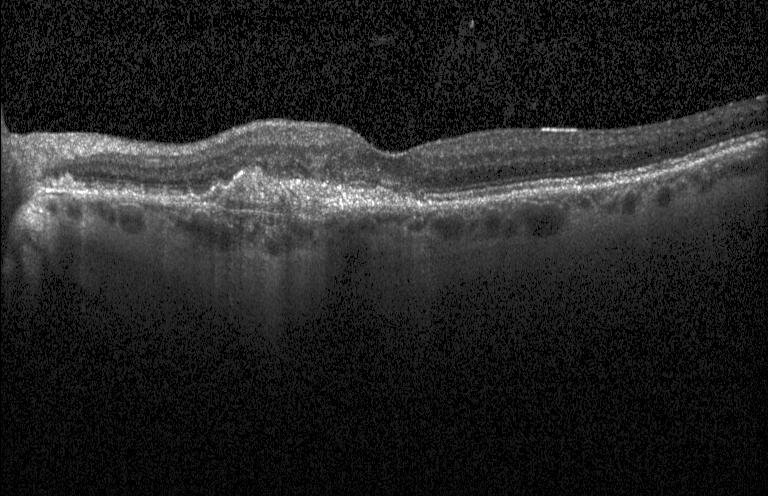

Diagnosis: choroidal neovascularization.